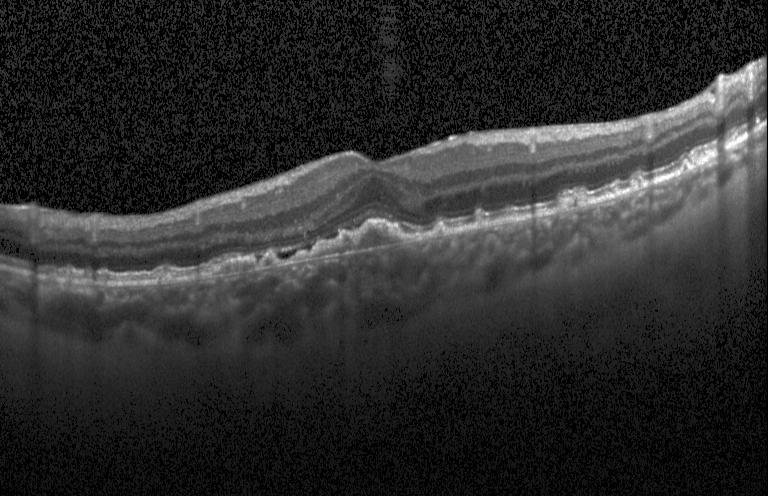
The scan shows choroidal neovascularization (CNV).